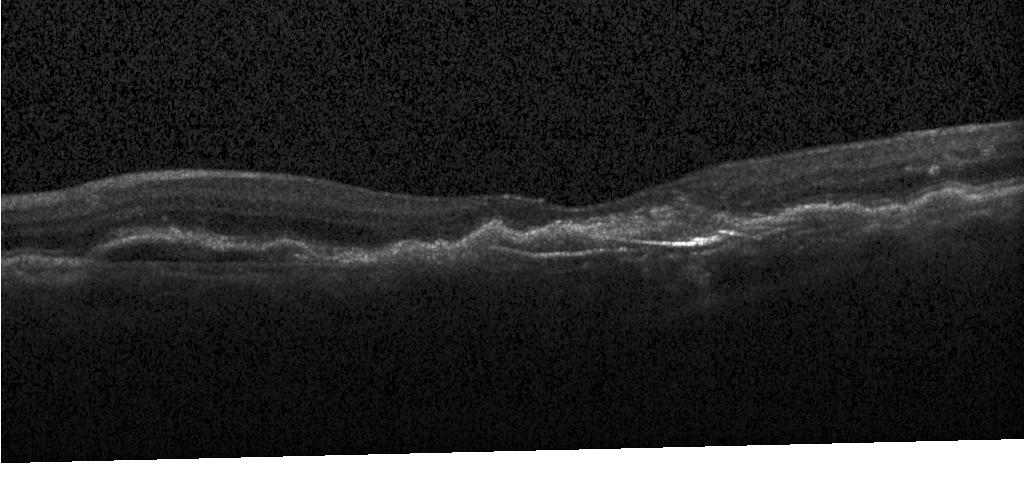
Retinal OCT cross-section. Macular OCT: a choroidal neovascular membrane.